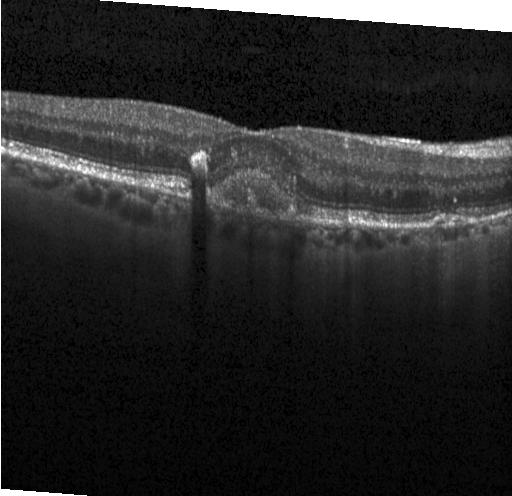
Diagnosis: a choroidal neovascular membrane.